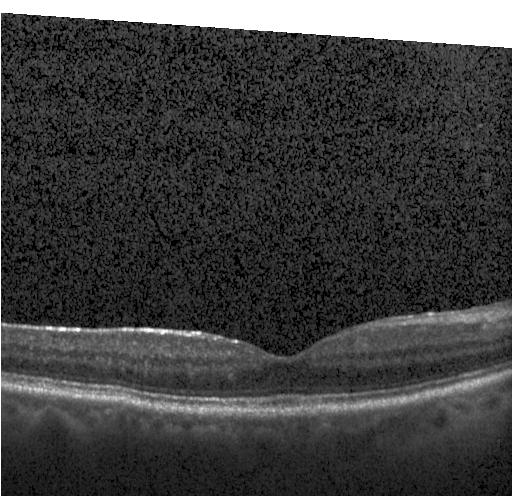

Instrument: Heidelberg Spectralis, through the macula, retinal OCT cross-section, spectral-domain OCT — The scan shows no choroidal neovascularization, diabetic macular edema, or drusen.